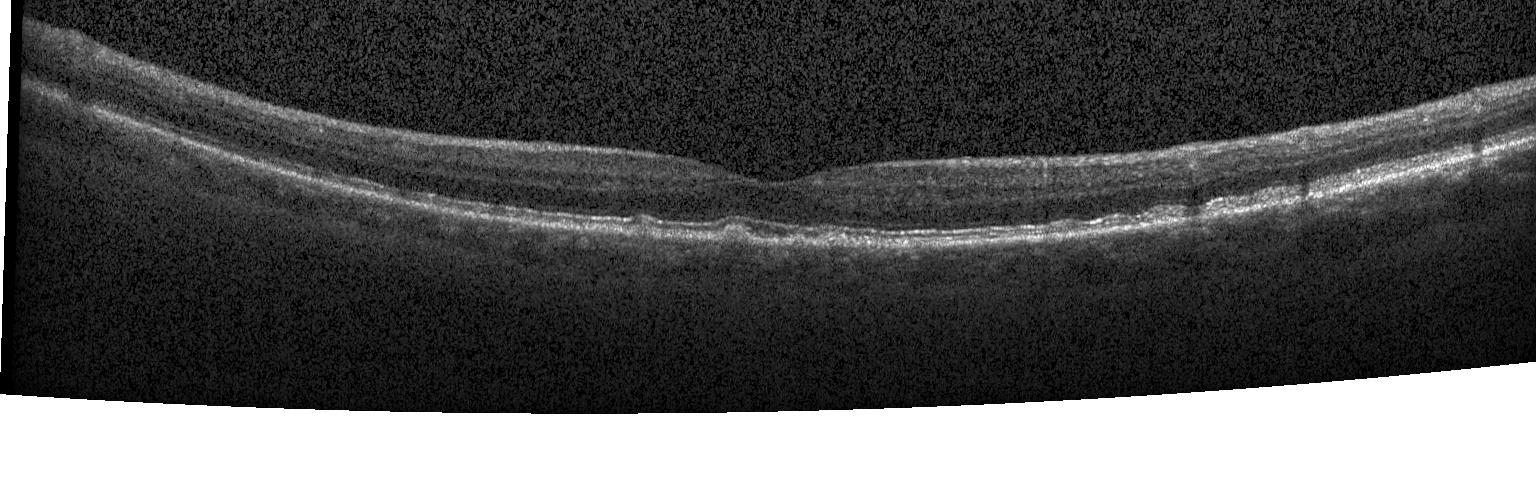 Spectral-domain optical coherence tomography, acquired on a Heidelberg Spectralis, retinal OCT B-scan.
OCT finding: drusen.